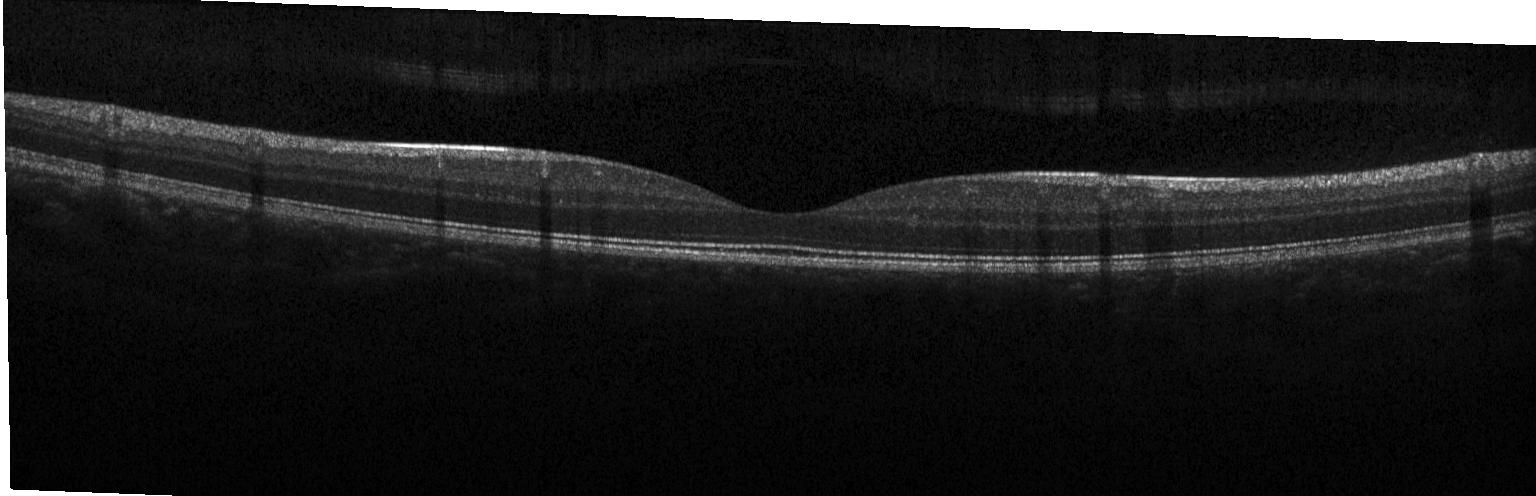 Spectral-domain OCT. Instrument: Heidelberg Spectralis. Macular scan. OCT B-scan — No choroidal neovascularization, no diabetic macular edema, and no drusen.